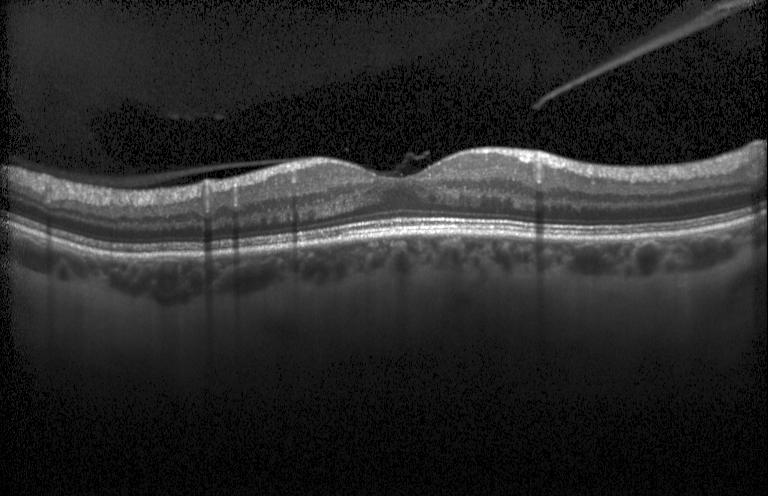

OCT finding: no choroidal neovascularization, diabetic macular edema, or drusen.